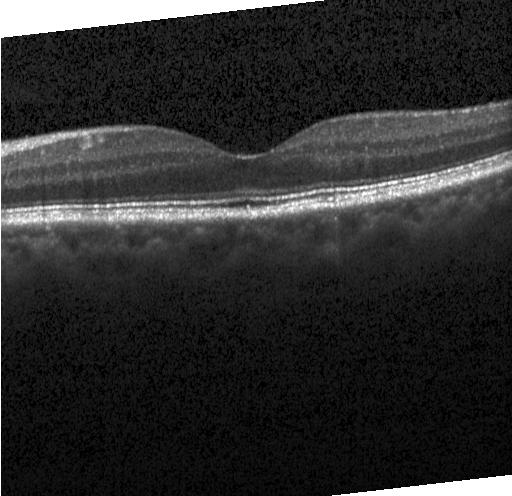 OCT B-scan · through the macula · instrument: Heidelberg Spectralis · SD-OCT
This B-scan demonstrates no choroidal neovascularization, no diabetic macular edema, and no drusen.